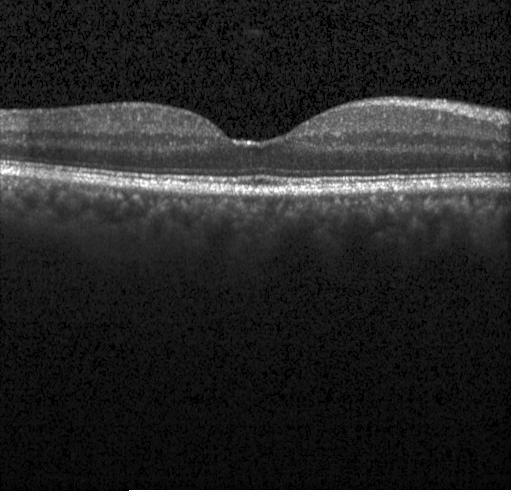
Assessment: no evidence of CNV, DME, or drusen.